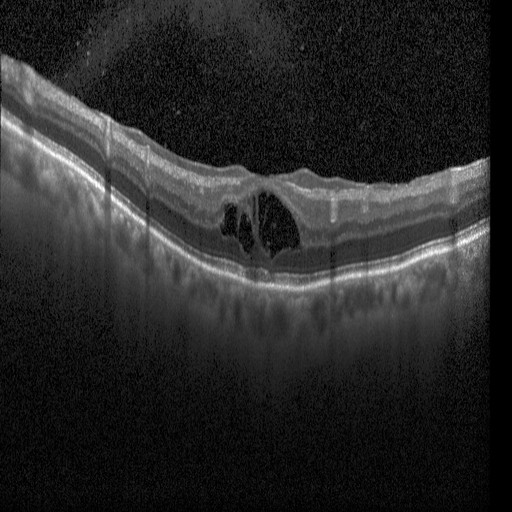

OCT B-scan. SD-OCT — DME.